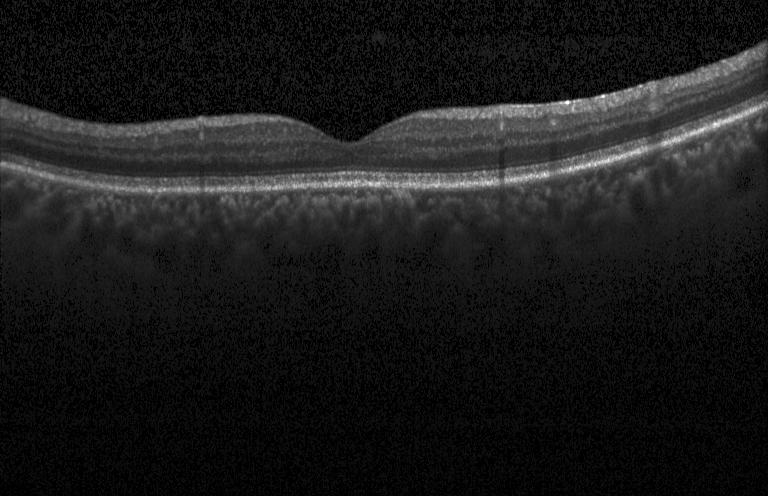

Centered on the fovea; retinal OCT cross-section; spectral-domain OCT. Finding: neither choroidal neovascularization, diabetic macular edema, nor drusen.